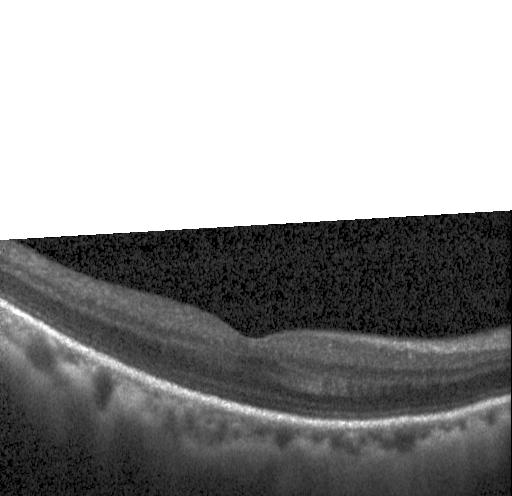 SD-OCT · retinal OCT B-scan · Heidelberg Spectralis OCT system
Assessment: no CNV, no DME, and no drusen.